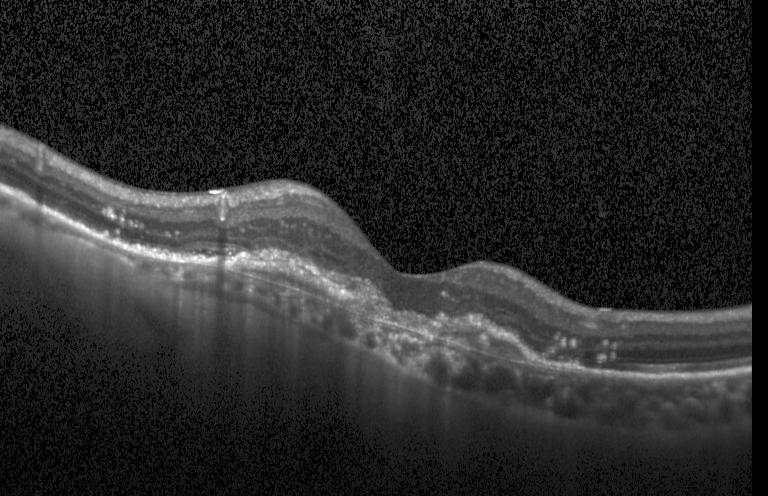 OCT line scan · Heidelberg Spectralis.
Impression: choroidal neovascularization.